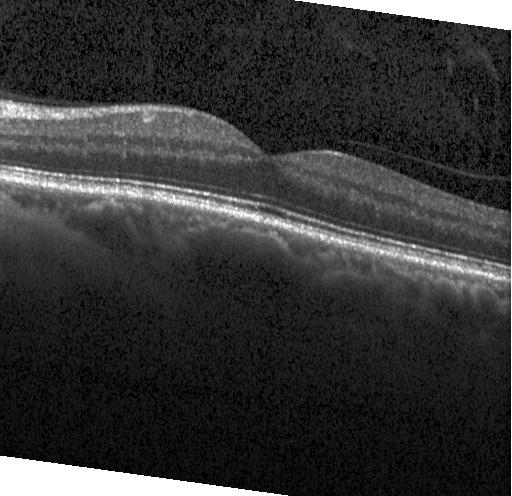

Finding: no choroidal neovascularization, diabetic macular edema, or drusen.